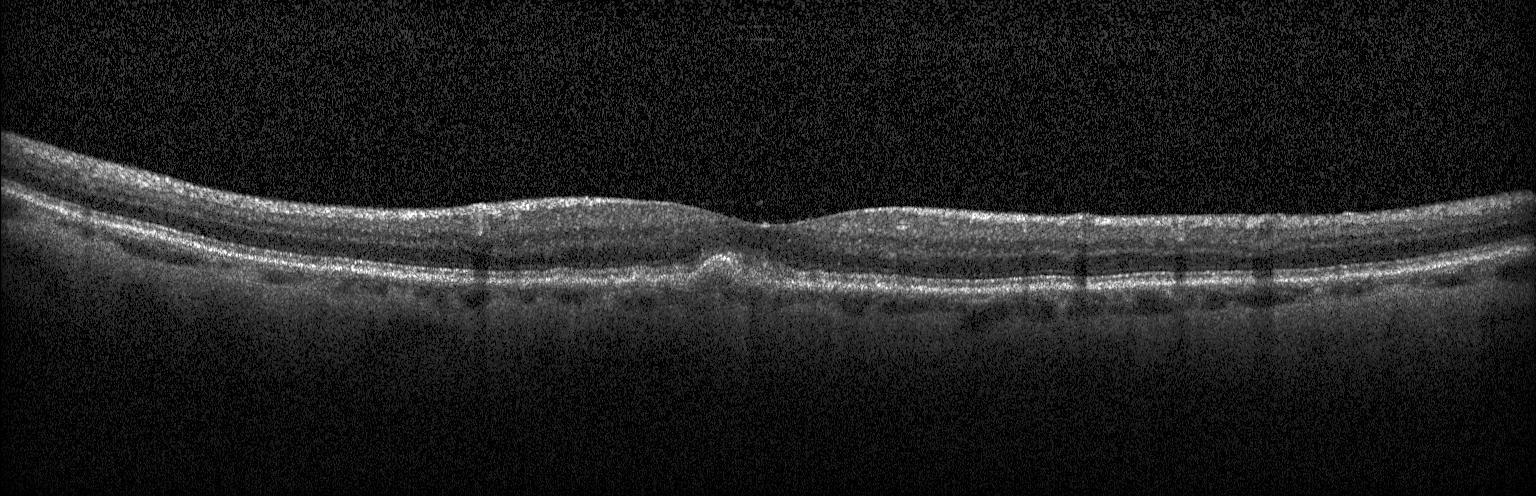
Retinal OCT cross-section — Assessment: sub-RPE drusenoid deposits.